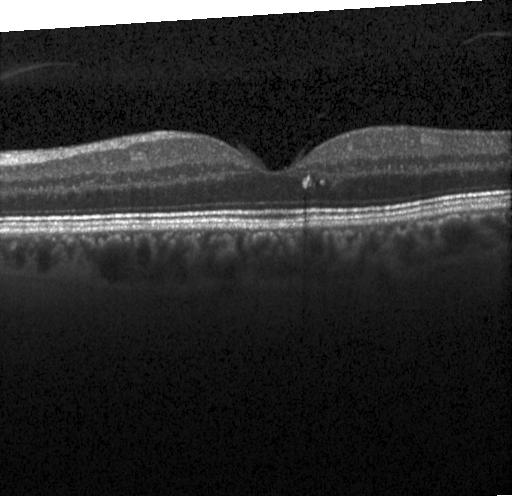

Finding: no choroidal neovascularization, diabetic macular edema, or drusen.